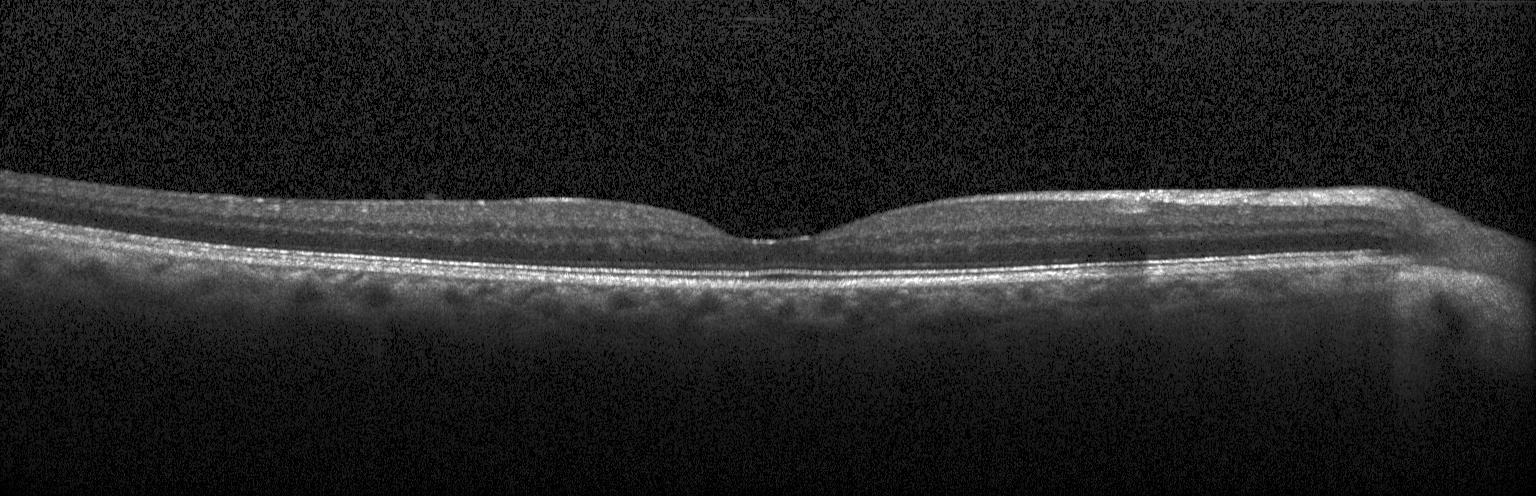
Spectral-domain optical coherence tomography · horizontal scan through the fovea · OCT B-scan — This B-scan demonstrates no evidence of choroidal neovascularization, diabetic macular edema, or drusen.